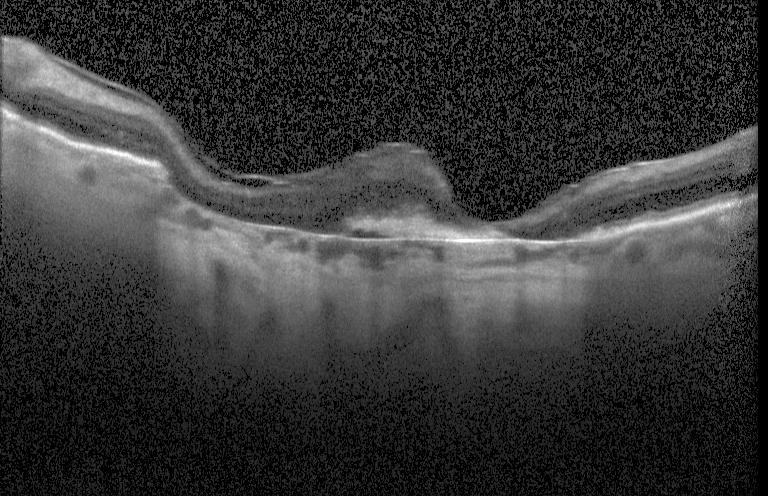

Impression: choroidal neovascularization (CNV).